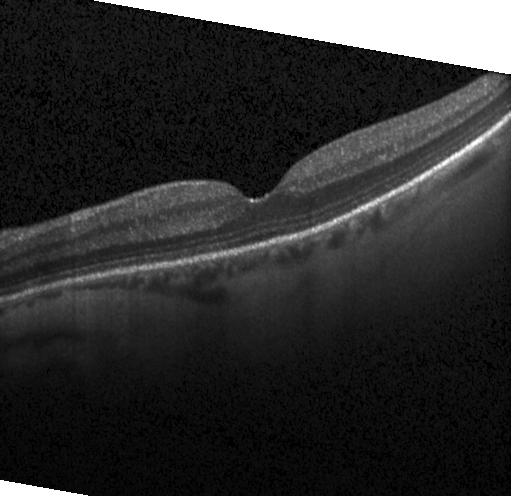
No evidence of choroidal neovascularization, diabetic macular edema, or drusen.